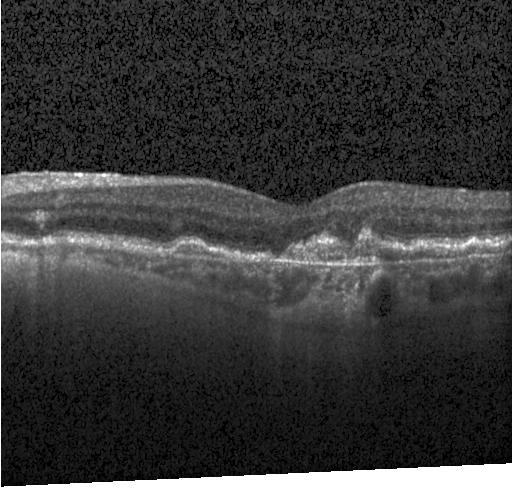 Finding: choroidal neovascularization (CNV).